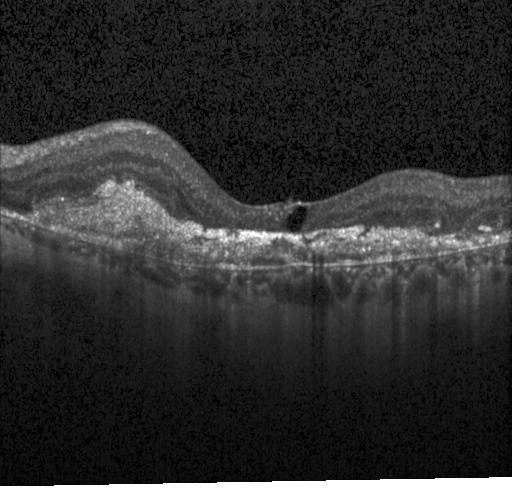
Retinal OCT B-scan.
Impression: choroidal neovascularization.